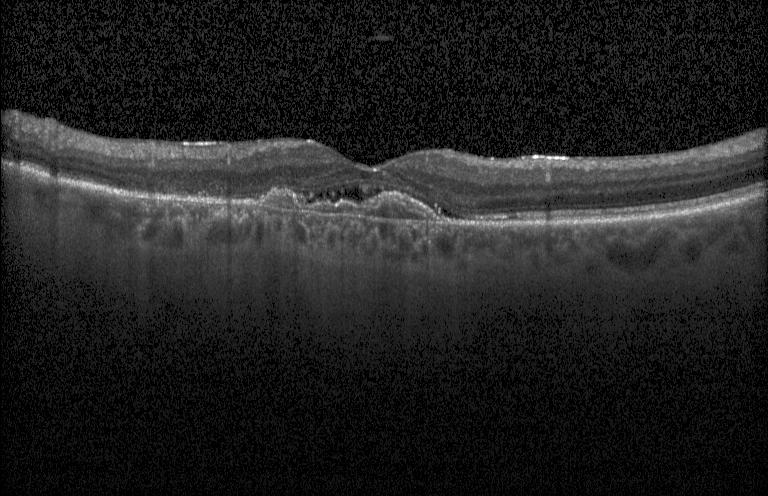
Optical coherence tomography scan · horizontal scan through the fovea — Finding: a choroidal neovascular membrane.